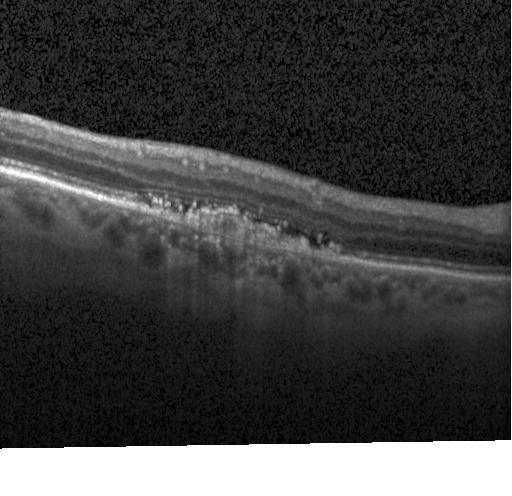
Heidelberg Spectralis OCT system; optical coherence tomography B-scan — A choroidal neovascular membrane.